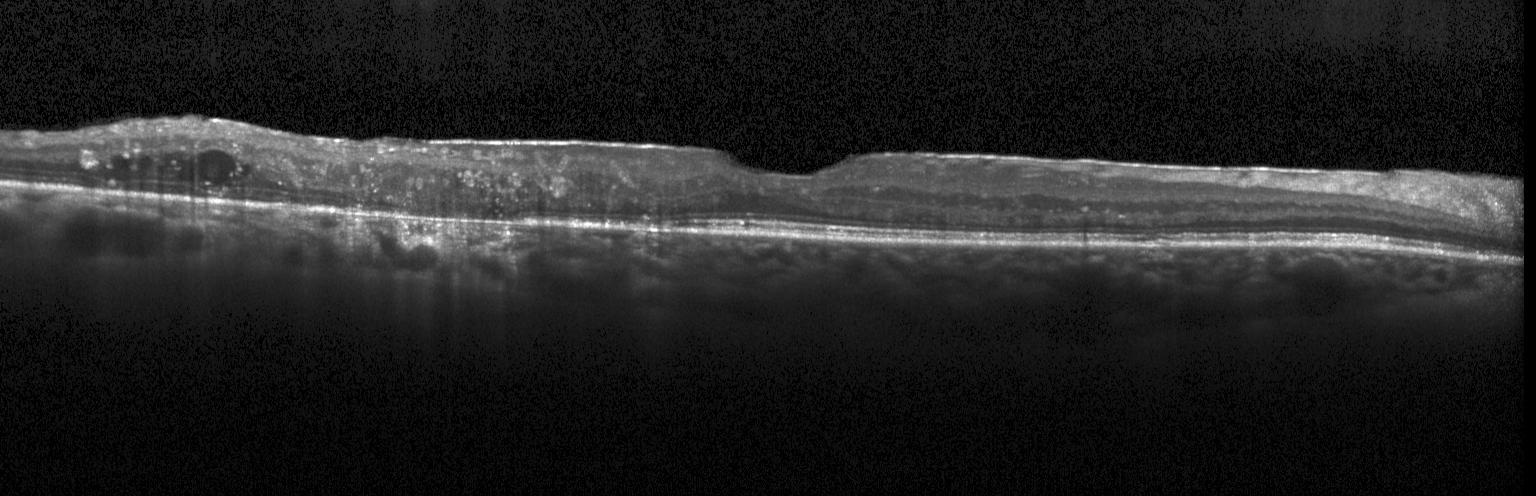
Retinal OCT cross-section. Assessment: diabetic macular edema (DME).